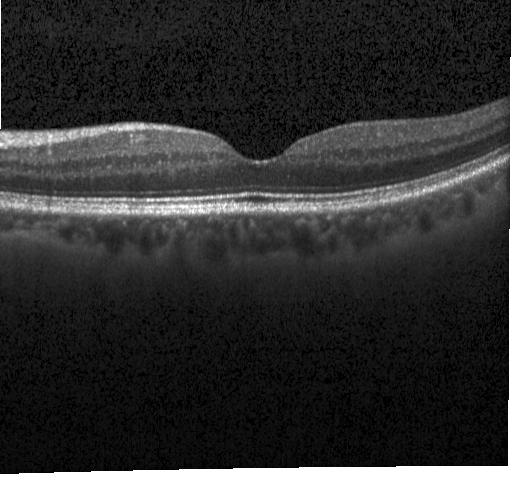 Centered on the fovea; acquired on a Heidelberg Spectralis; retinal OCT cross-section
No choroidal neovascularization, no diabetic macular edema, and no drusen.